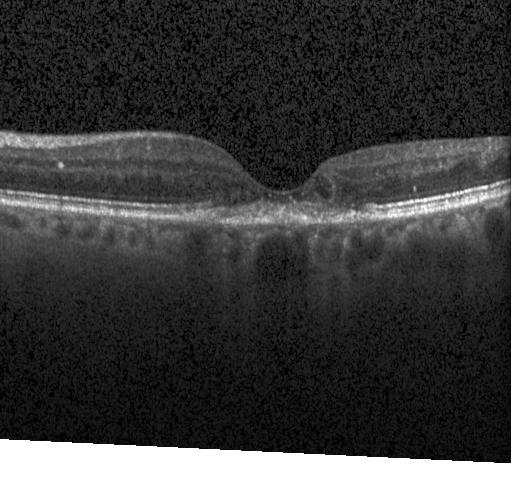 OCT B-scan; Heidelberg Spectralis OCT system
Impression: a choroidal neovascular membrane.